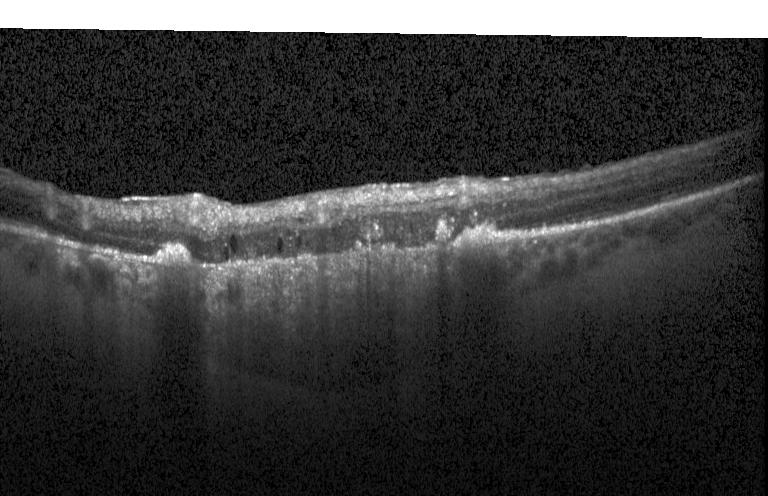

OCT finding: choroidal neovascularization (CNV).